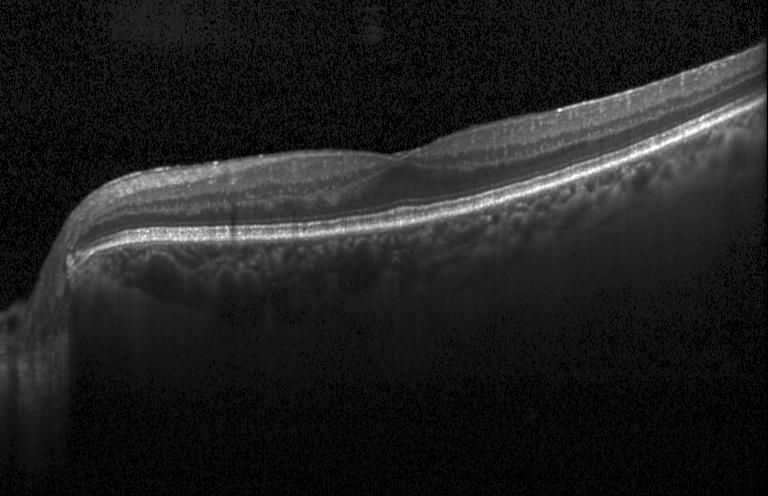
Retinal OCT B-scan — This B-scan demonstrates no CNV, no DME, and no drusen.